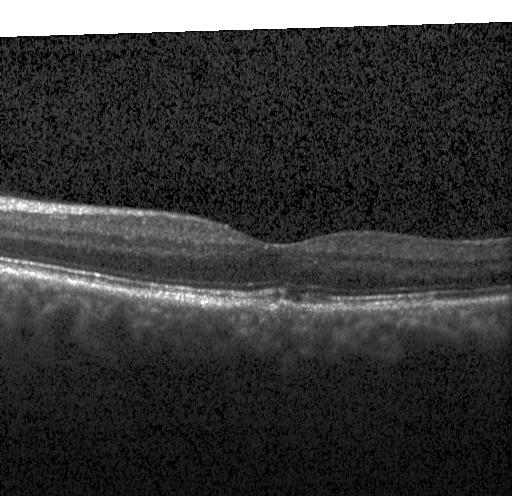 Instrument: Heidelberg Spectralis · optical coherence tomography scan · spectral-domain OCT. Drusen.